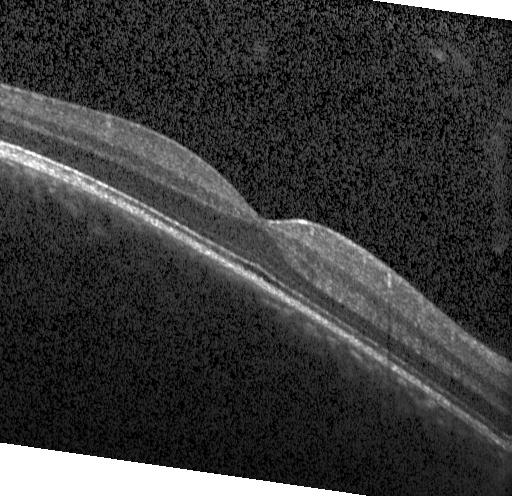

Retinal OCT cross-section. Horizontal scan through the fovea. Spectral-domain optical coherence tomography. Heidelberg Spectralis OCT system.
OCT finding: no CNV, DME, or drusen.